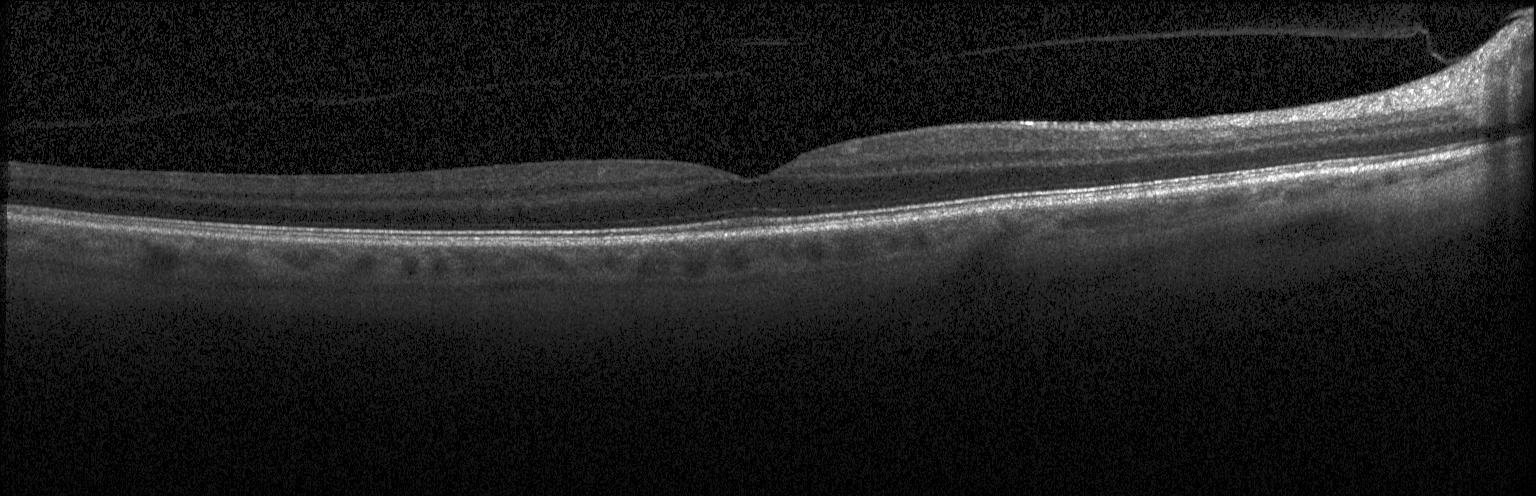 Optical coherence tomography B-scan. OCT finding: no choroidal neovascularization, no diabetic macular edema, and no drusen.